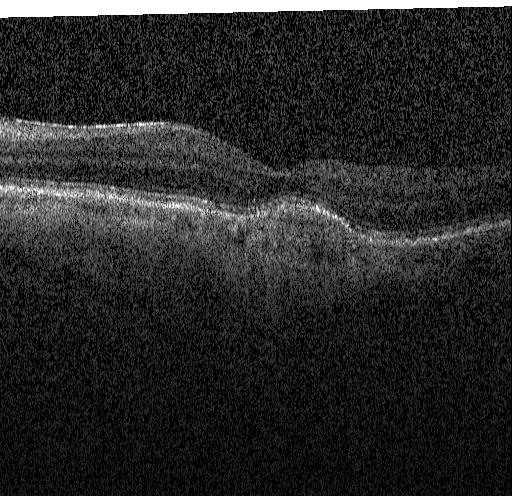
Impression: a choroidal neovascular membrane.